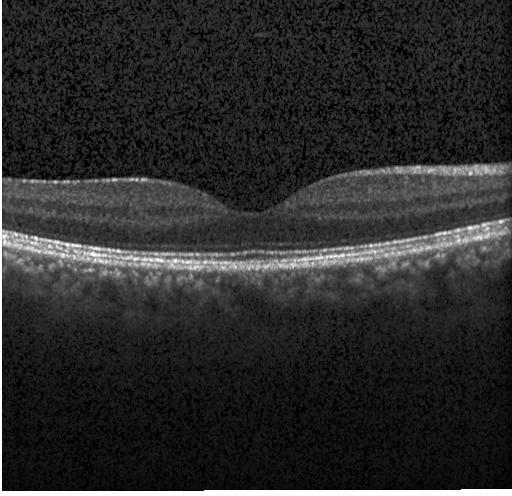

Macular scan, OCT line scan.
Finding: no CNV, no DME, and no drusen.